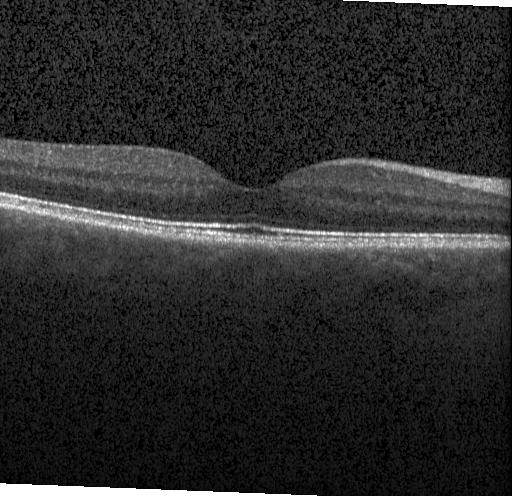 Spectral-domain OCT, centered on the fovea, Heidelberg Spectralis, OCT line scan.
OCT finding: no CNV, no DME, and no drusen.